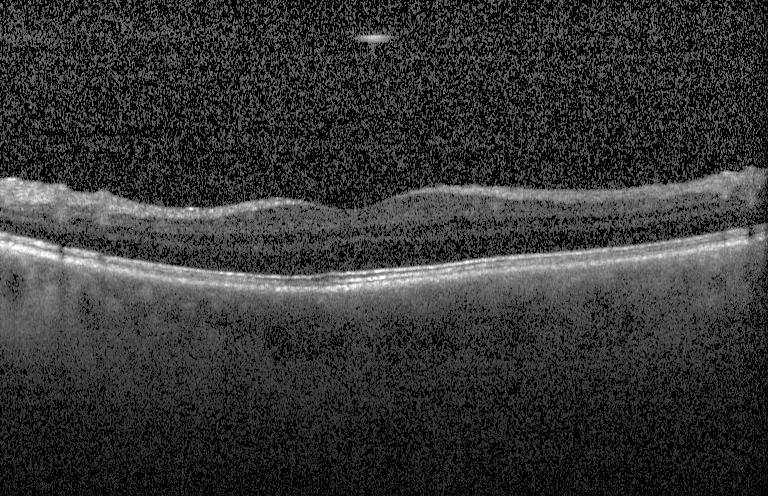
OCT B-scan showing no CNV, no DME, and no drusen.